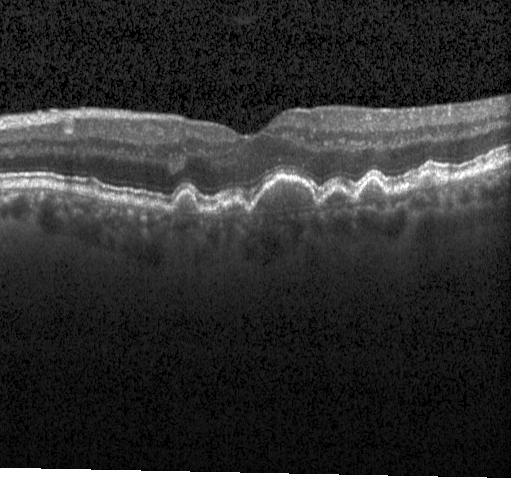
OCT scan showing multiple drusen.